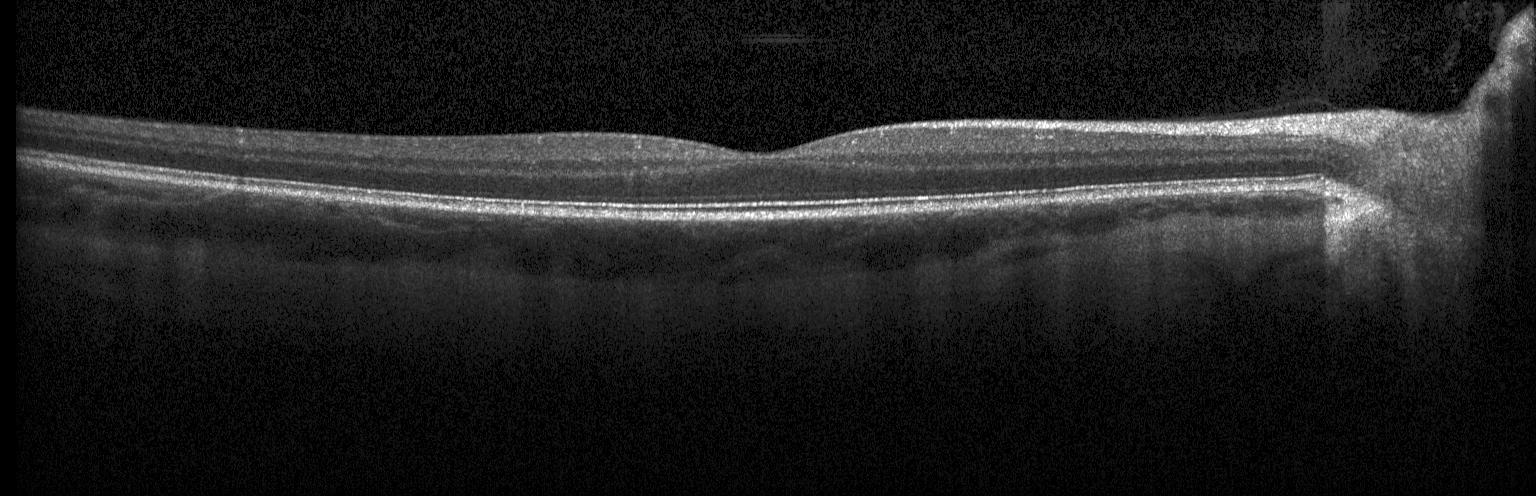

Optical coherence tomography scan; spectral-domain OCT; fovea-centered
Impression: no choroidal neovascularization, diabetic macular edema, or drusen.